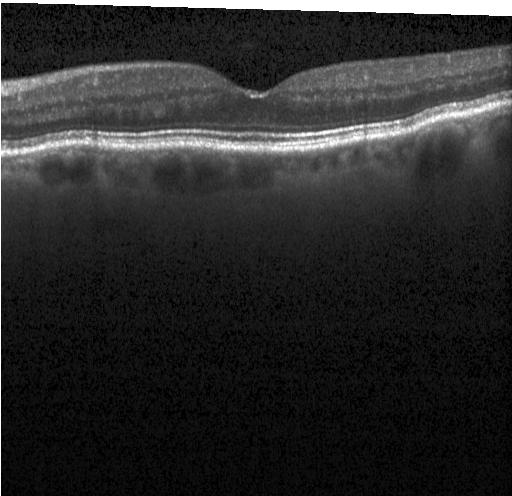
Retinal OCT cross-section · acquired on a Heidelberg Spectralis
Finding: no evidence of CNV, DME, or drusen.